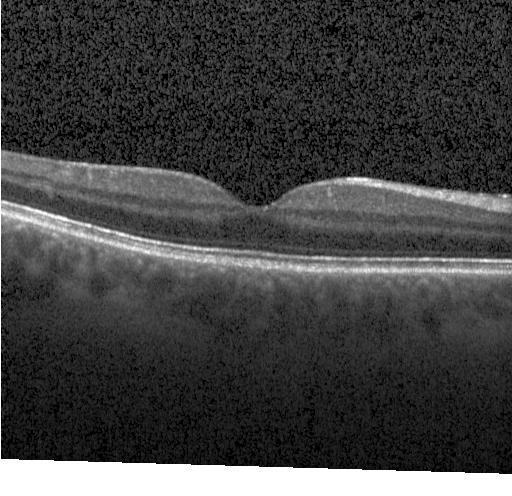

Finding: no choroidal neovascularization, diabetic macular edema, or drusen.